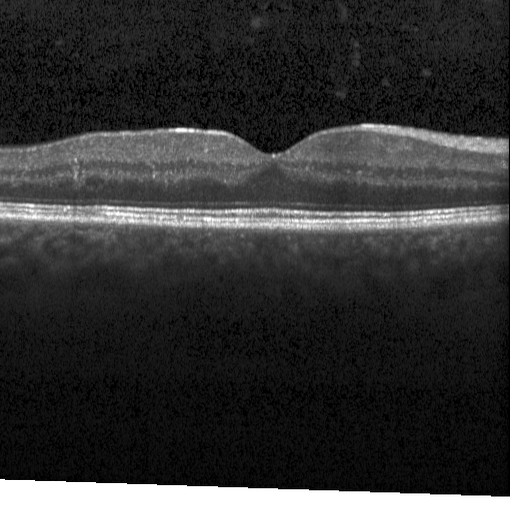
Finding: diabetic macular edema (DME).